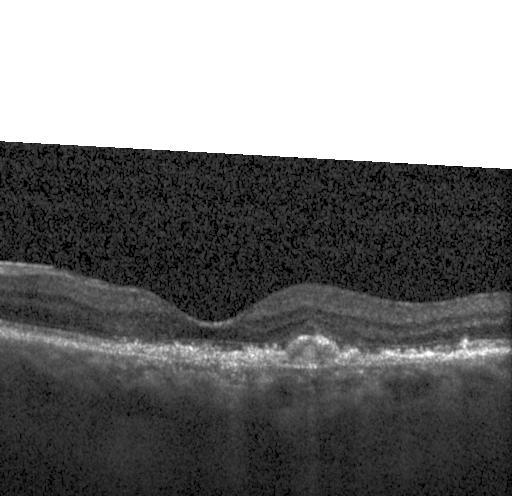 Heidelberg Spectralis OCT system, OCT B-scan, spectral-domain optical coherence tomography
Diagnosis: a choroidal neovascular membrane.